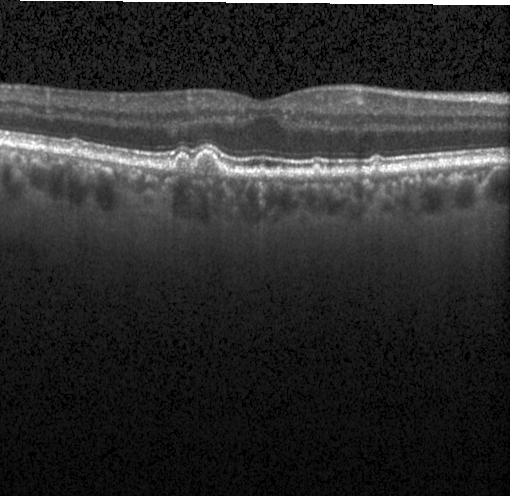 Optical coherence tomography scan, spectral-domain optical coherence tomography. Impression: multiple drusen.